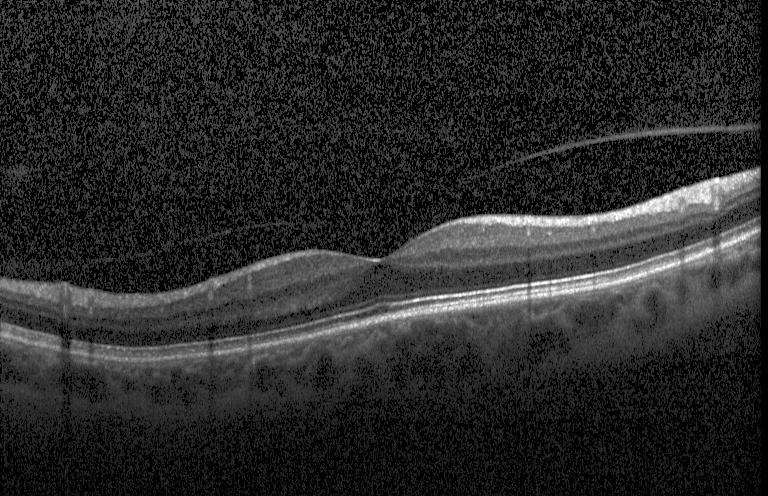
Dx: no evidence of CNV, DME, or drusen.